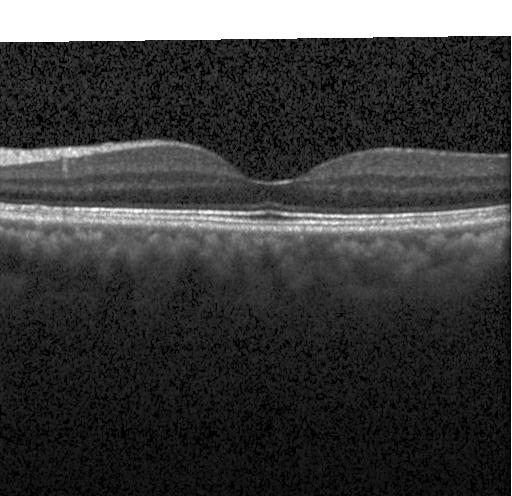 Optical coherence tomography B-scan, horizontal scan through the fovea, acquired on a Heidelberg Spectralis.
Finding: neither choroidal neovascularization, diabetic macular edema, nor drusen.